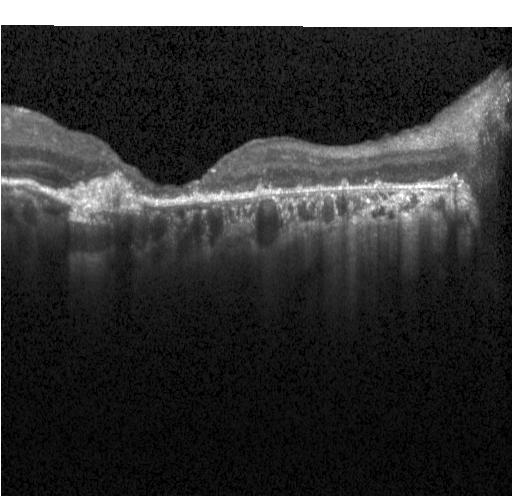
Retinal OCT cross-section.
Finding: a choroidal neovascular membrane.